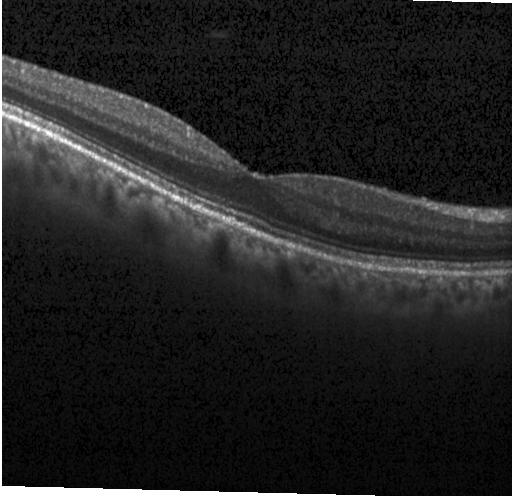 Optical coherence tomography B-scan; Heidelberg Spectralis OCT system — This B-scan demonstrates no CNV, no DME, and no drusen.